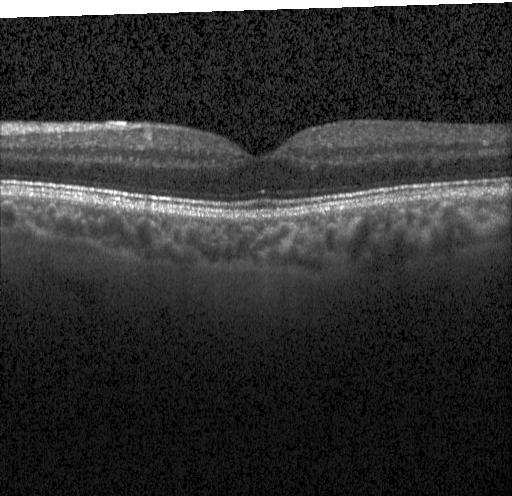
This B-scan demonstrates neither CNV, DME, nor drusen.